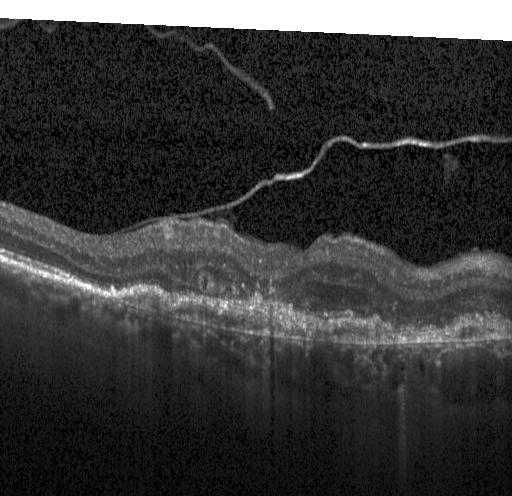 Optical coherence tomography B-scan; spectral-domain OCT; Heidelberg Spectralis OCT system — Impression: a choroidal neovascular membrane.